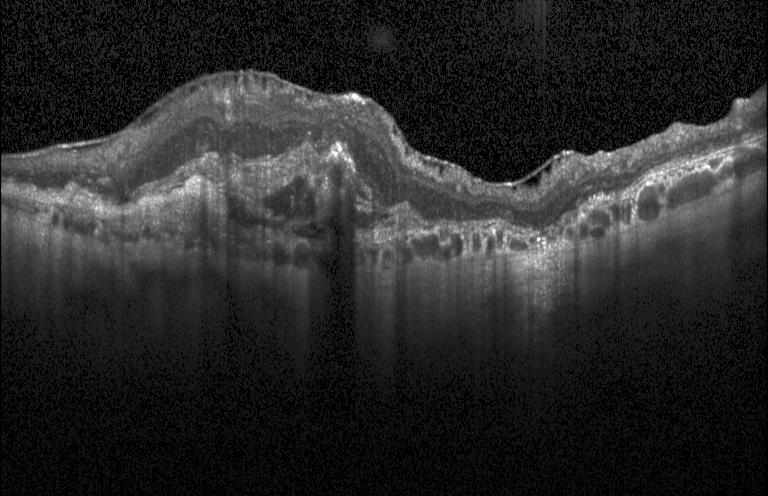 OCT B-scan. Macular scan
Dx: a choroidal neovascular membrane.